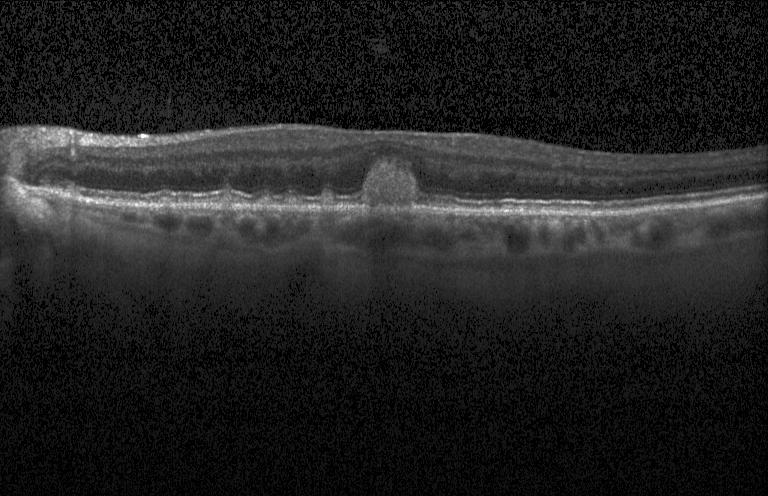

SD-OCT; instrument: Heidelberg Spectralis; macular scan; retinal OCT B-scan. OCT finding: a choroidal neovascular membrane.